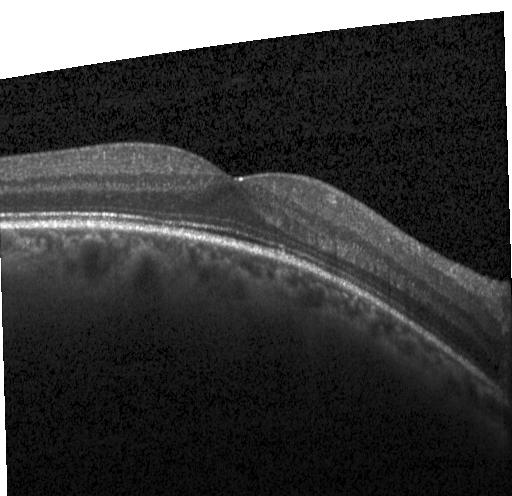 OCT B-scan. Heidelberg Spectralis OCT system
Finding: no choroidal neovascularization, no diabetic macular edema, and no drusen.